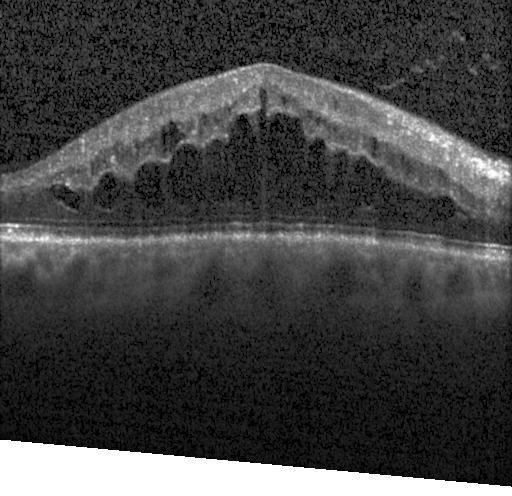

Spectral-domain OCT. Retinal OCT B-scan
Finding: diabetic macular edema.